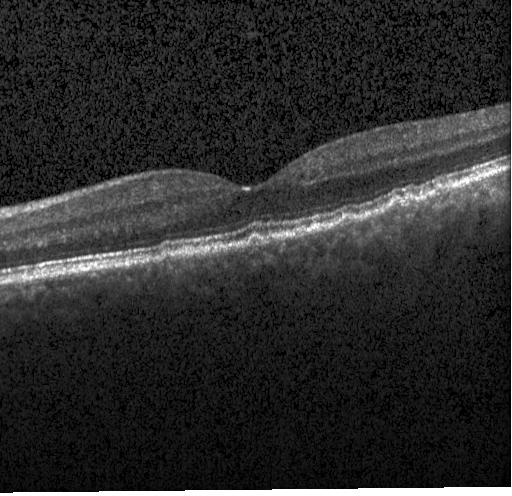
Diagnosis: sub-RPE drusenoid deposits.